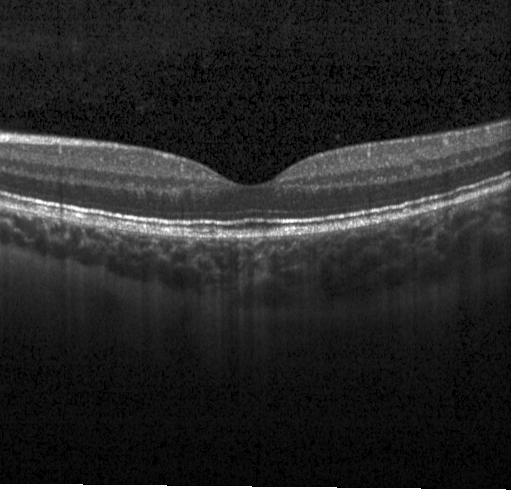
Retinal OCT cross-section; through the macula; Heidelberg Spectralis OCT system; spectral-domain OCT
Impression: neither choroidal neovascularization, diabetic macular edema, nor drusen.